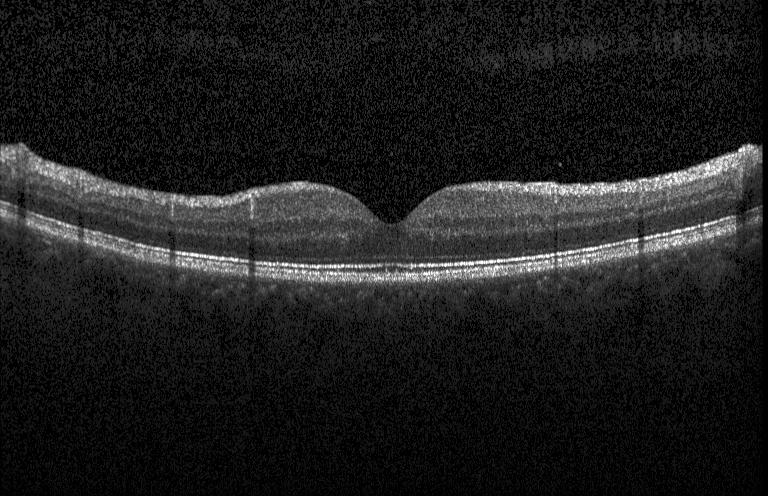 Spectral-domain optical coherence tomography; fovea-centered; OCT B-scan.
No choroidal neovascularization, diabetic macular edema, or drusen.